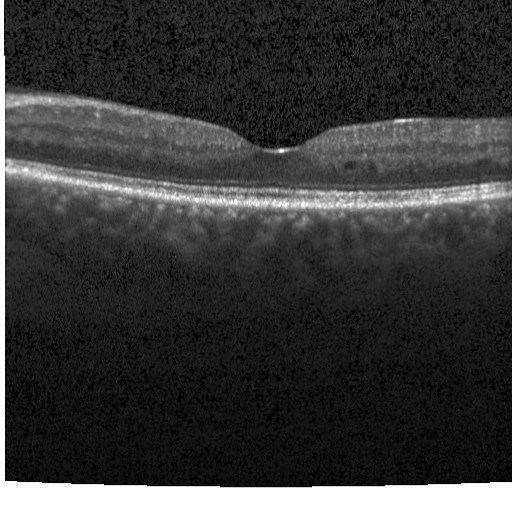

Finding: diabetic macular edema (DME).